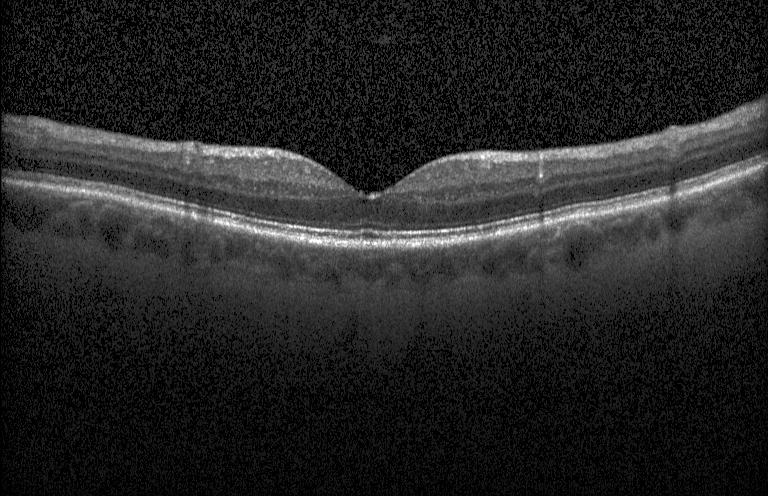 Macular OCT: no choroidal neovascularization, no diabetic macular edema, and no drusen.